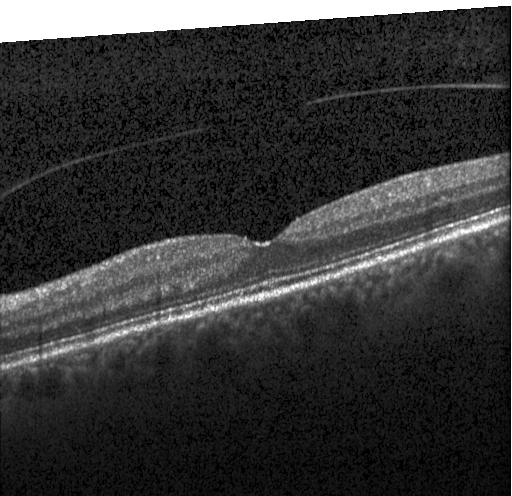
Horizontal scan through the fovea; optical coherence tomography B-scan — Diagnosis: no CNV, no DME, and no drusen.